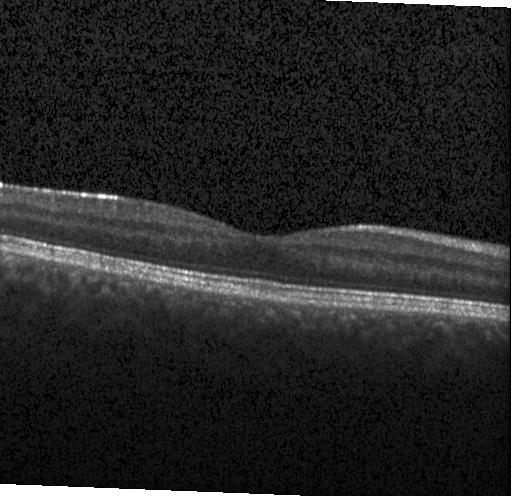 Diagnosis: no choroidal neovascularization, diabetic macular edema, or drusen.